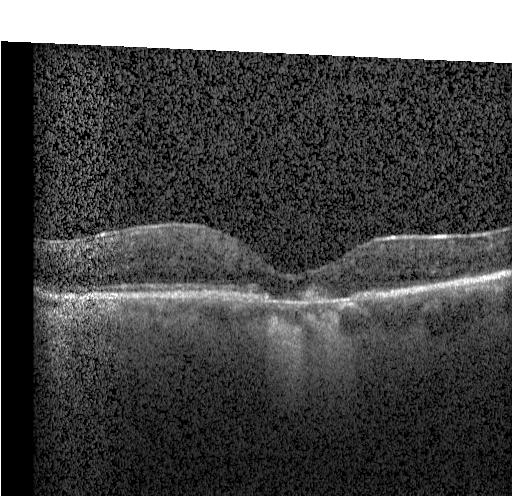
Centered on the fovea. Heidelberg Spectralis OCT system. Retinal OCT cross-section. SD-OCT
Assessment: CNV.